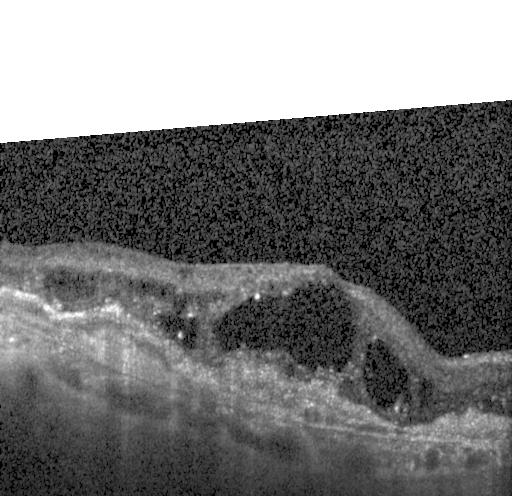 Macular scan; optical coherence tomography scan; spectral-domain optical coherence tomography; Heidelberg Spectralis OCT system — Finding: a choroidal neovascular membrane.